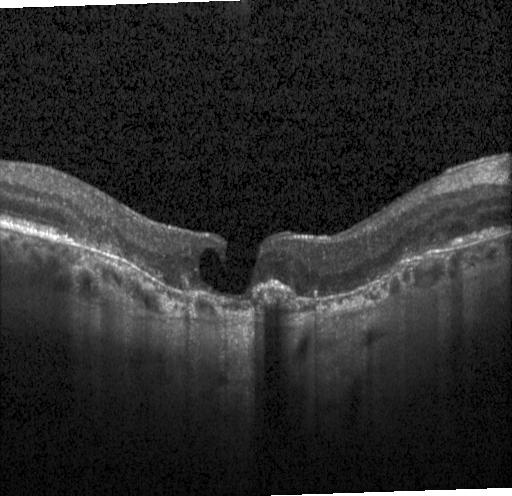
Through the macula; instrument: Heidelberg Spectralis; optical coherence tomography B-scan; SD-OCT — Impression: a choroidal neovascular membrane.